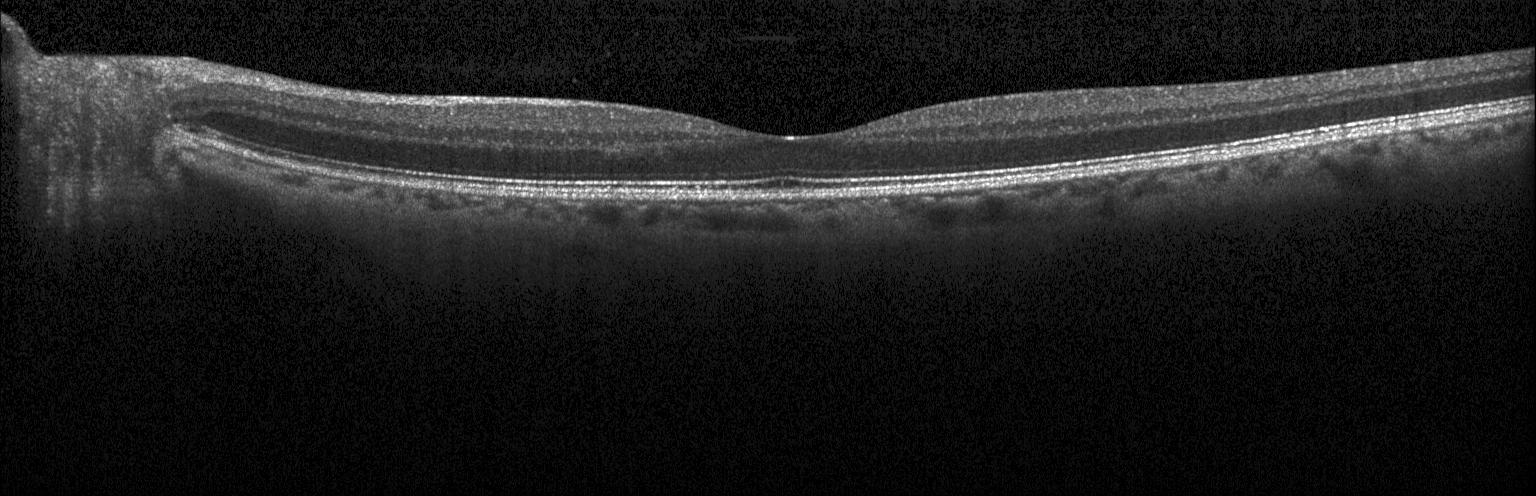

Diagnosis: no CNV, DME, or drusen.